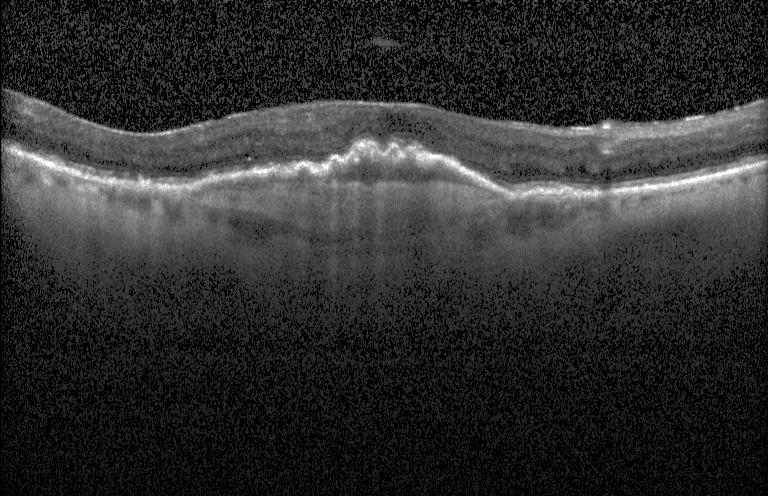

Macular scan. Optical coherence tomography B-scan.
Finding: CNV.